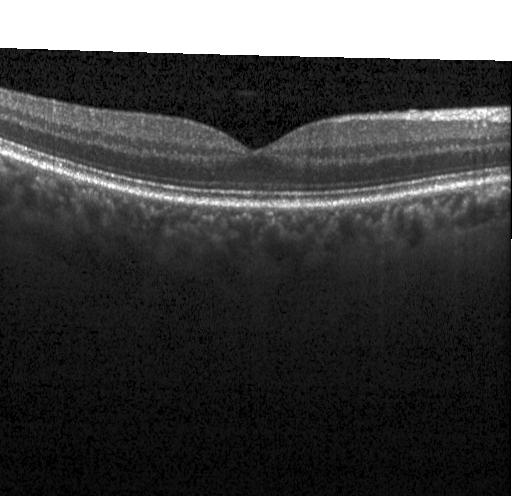

Instrument: Heidelberg Spectralis. Optical coherence tomography B-scan. Impression: neither CNV, DME, nor drusen.